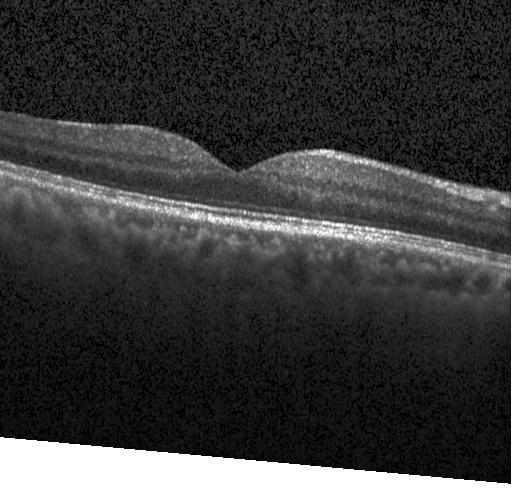

OCT scan showing no evidence of choroidal neovascularization, diabetic macular edema, or drusen.